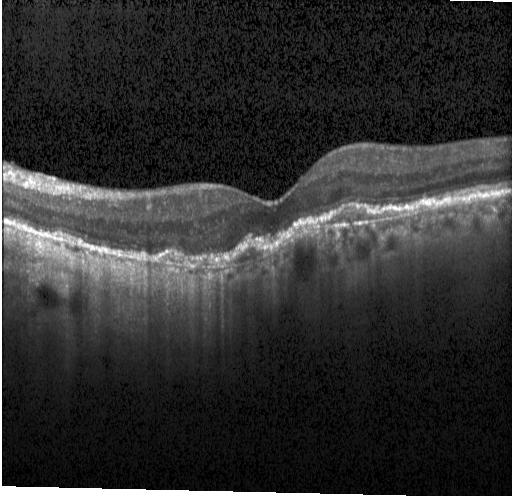
Optical coherence tomography B-scan. Diagnosis: a choroidal neovascular membrane.